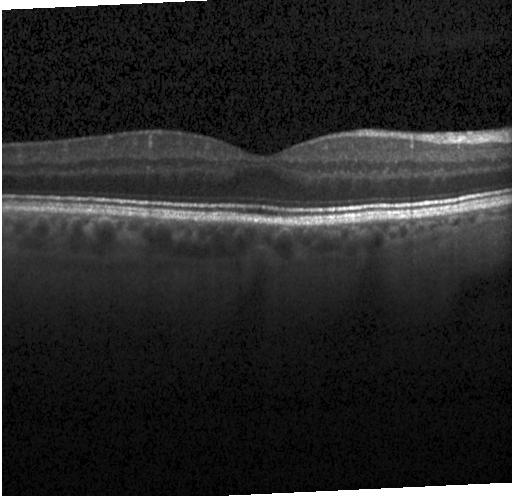 The scan shows no evidence of choroidal neovascularization, diabetic macular edema, or drusen.